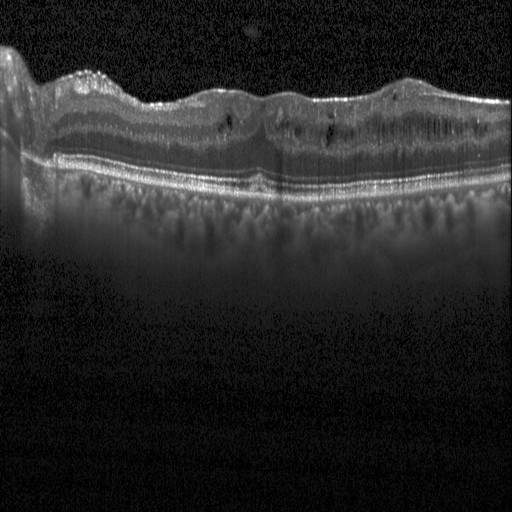
Retinal OCT cross-section showing diabetic macular edema (DME).